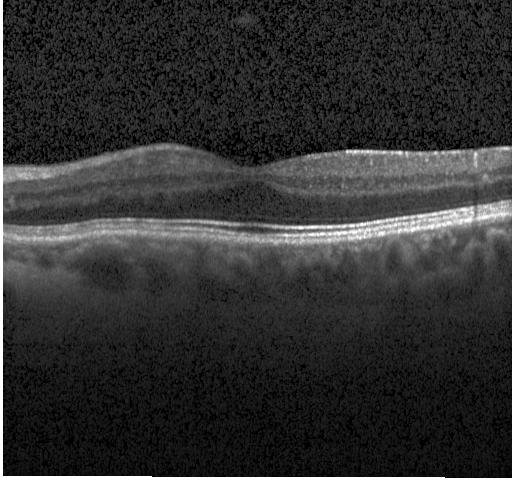
Heidelberg Spectralis OCT system · spectral-domain OCT · horizontal scan through the fovea · retinal OCT cross-section
Finding: no evidence of choroidal neovascularization, diabetic macular edema, or drusen.